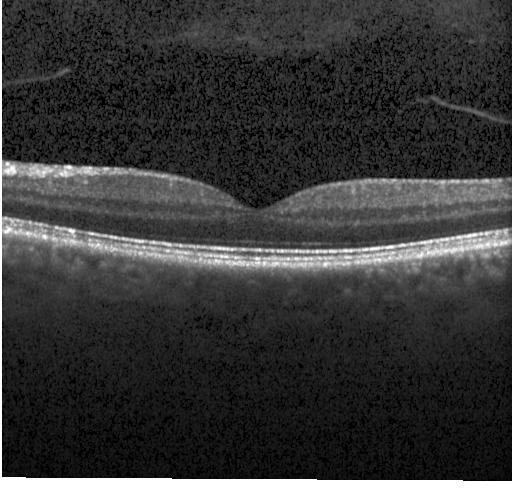
Optical coherence tomography scan. Heidelberg Spectralis OCT system. Centered on the fovea.
Macular OCT: neither CNV, DME, nor drusen.